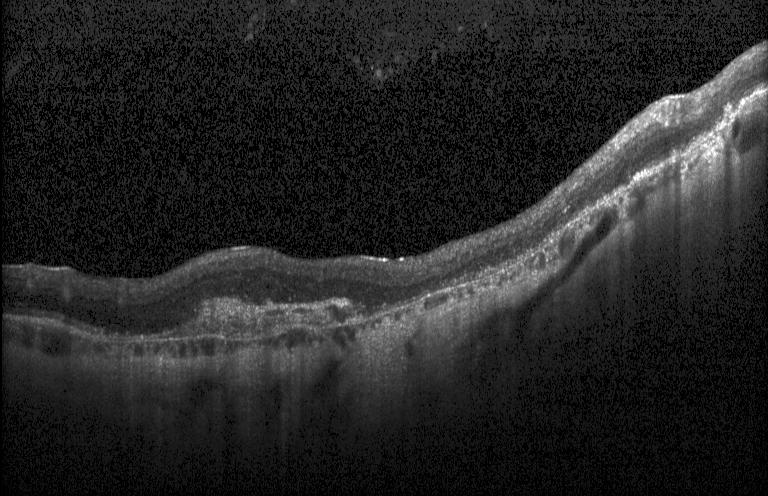
Macular OCT: CNV.